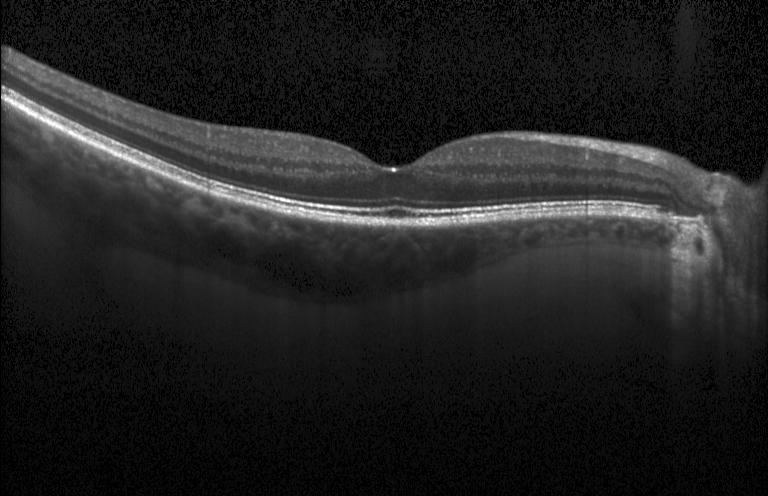 Retinal OCT cross-section; acquired on a Heidelberg Spectralis
The scan shows no evidence of choroidal neovascularization, diabetic macular edema, or drusen.